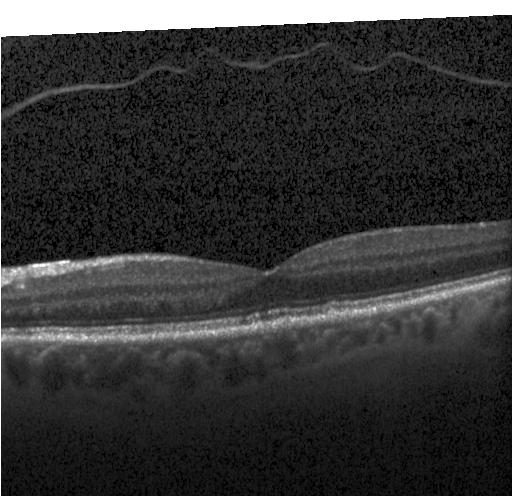 Instrument: Heidelberg Spectralis; fovea-centered; optical coherence tomography scan; spectral-domain optical coherence tomography
OCT finding: sub-RPE drusenoid deposits.